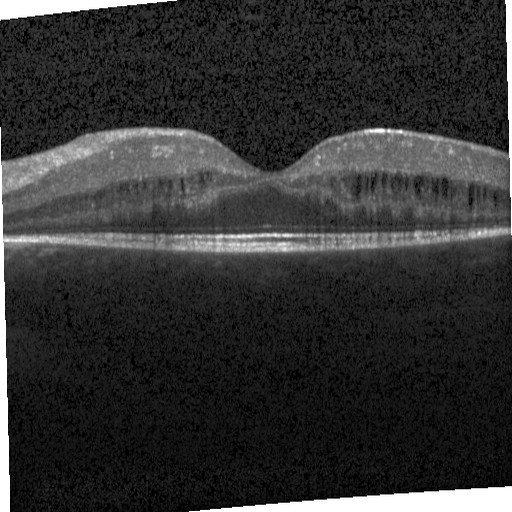

SD-OCT, retinal OCT cross-section, instrument: Heidelberg Spectralis, fovea-centered.
OCT finding: diabetic macular edema (DME).